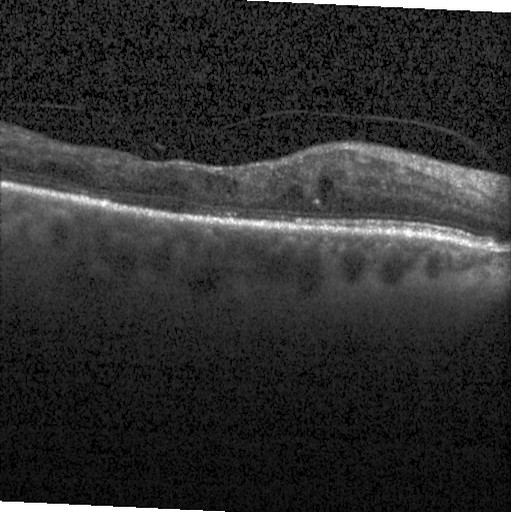 Retinal OCT B-scan; instrument: Heidelberg Spectralis; horizontal scan through the fovea.
Finding: DME.